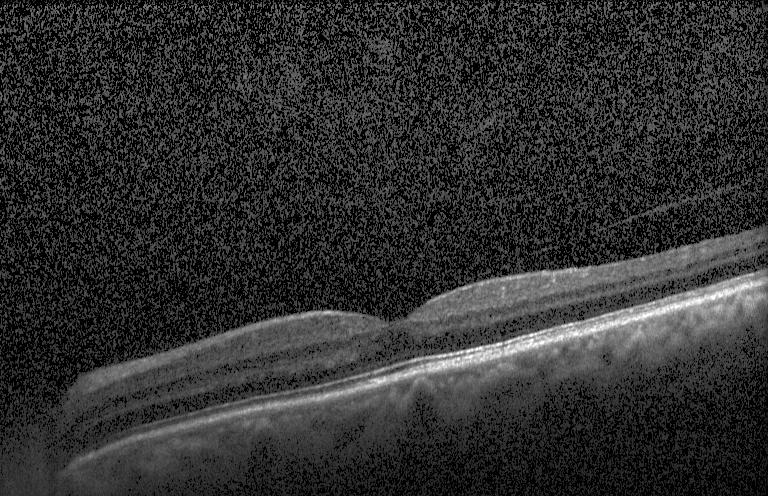

No CNV, no DME, and no drusen.